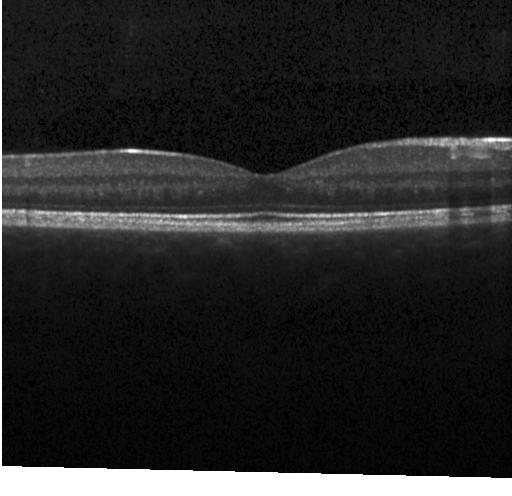 Heidelberg Spectralis OCT system. Through the macula. OCT B-scan. Spectral-domain OCT. The scan shows no choroidal neovascularization, diabetic macular edema, or drusen.